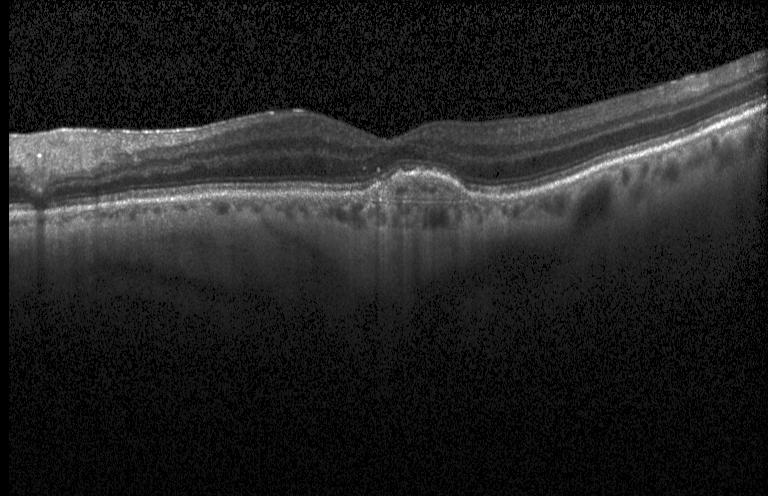 The scan shows a choroidal neovascular membrane.